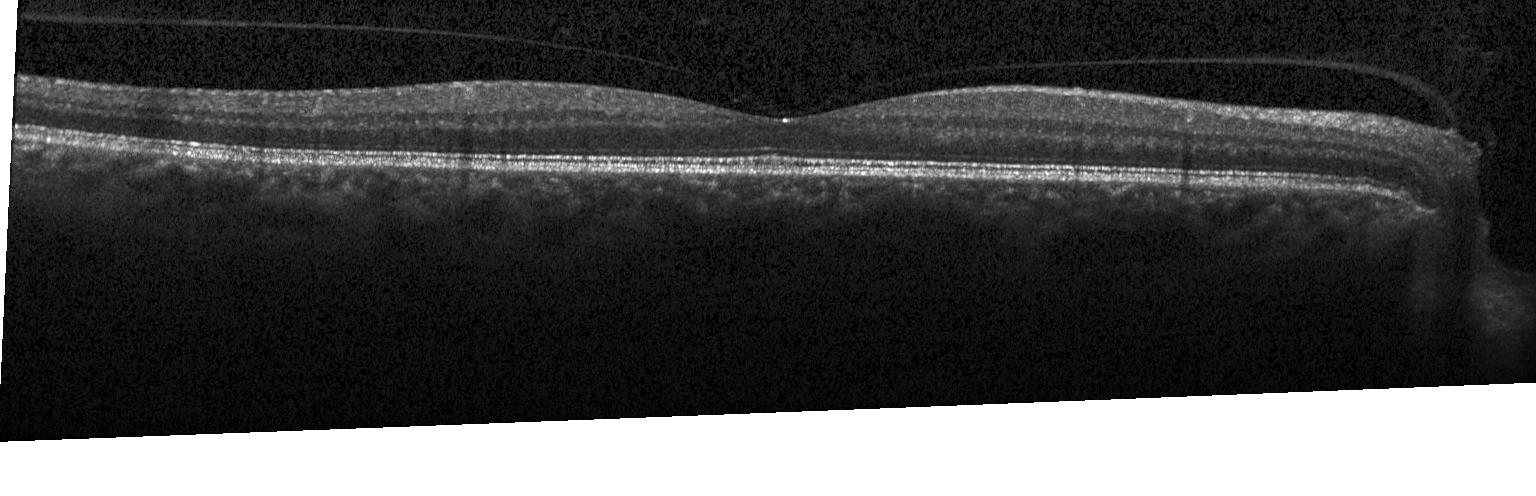
Optical coherence tomography scan; Heidelberg Spectralis
Finding: no CNV, DME, or drusen.